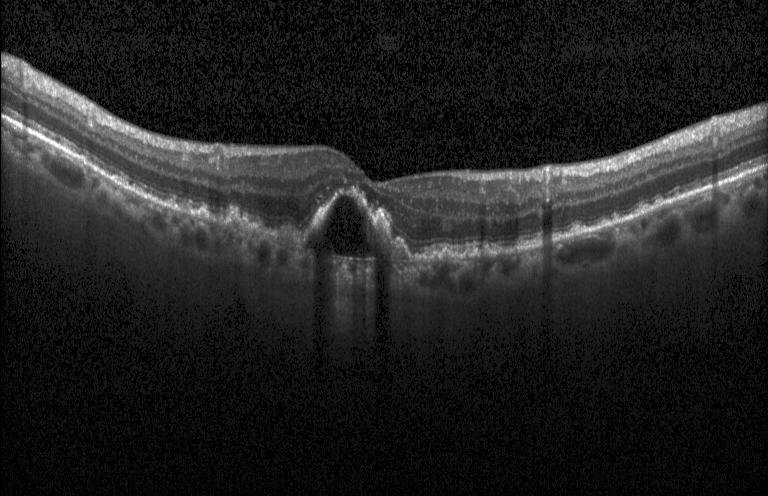
Retinal OCT cross-section showing choroidal neovascularization (CNV).